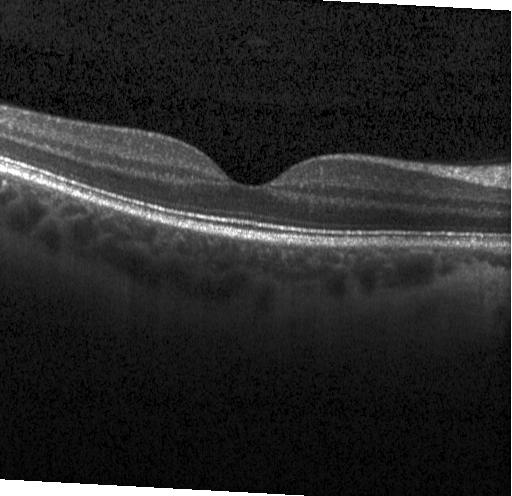 Macular scan · optical coherence tomography scan · SD-OCT · Heidelberg Spectralis. OCT finding: no evidence of choroidal neovascularization, diabetic macular edema, or drusen.